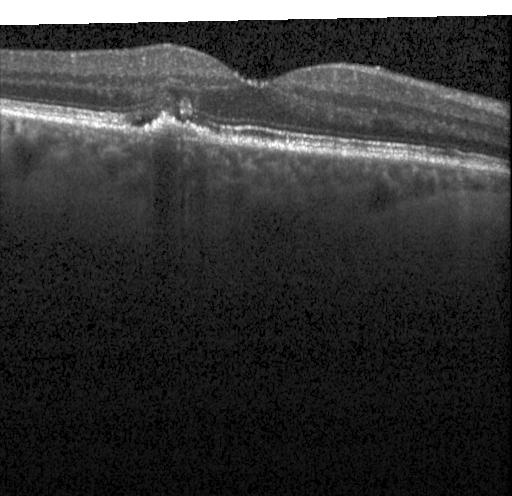

OCT line scan. Instrument: Heidelberg Spectralis. SD-OCT — Impression: choroidal neovascularization (CNV).